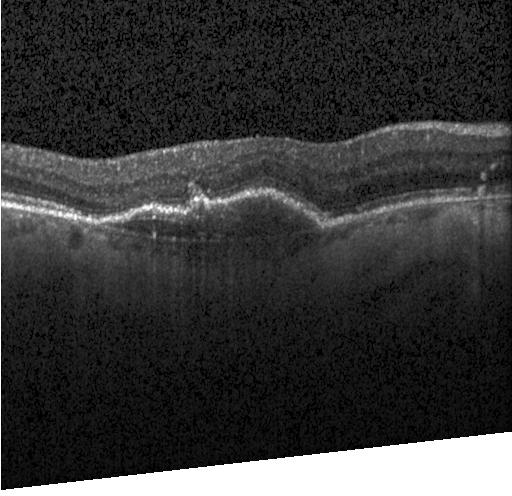 Optical coherence tomography scan · spectral-domain OCT · Heidelberg Spectralis OCT system · centered on the fovea. Finding: a choroidal neovascular membrane.